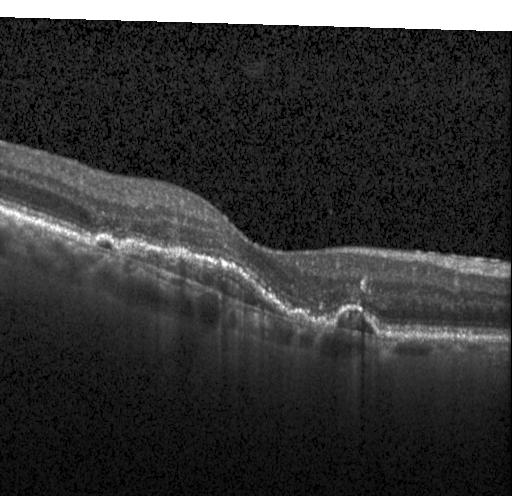
Dx: CNV.